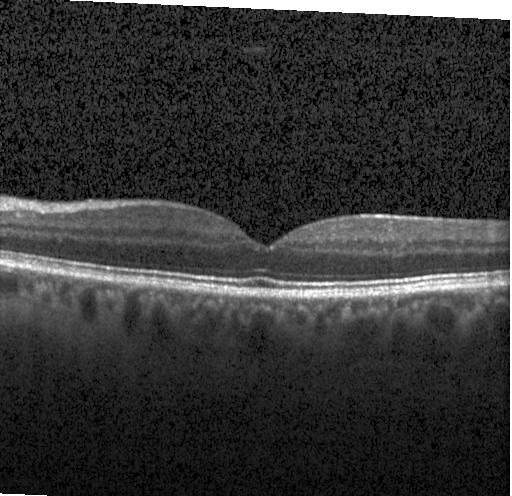 Horizontal scan through the fovea. Optical coherence tomography scan. Spectral-domain OCT. Heidelberg Spectralis OCT system. Diagnosis: neither CNV, DME, nor drusen.